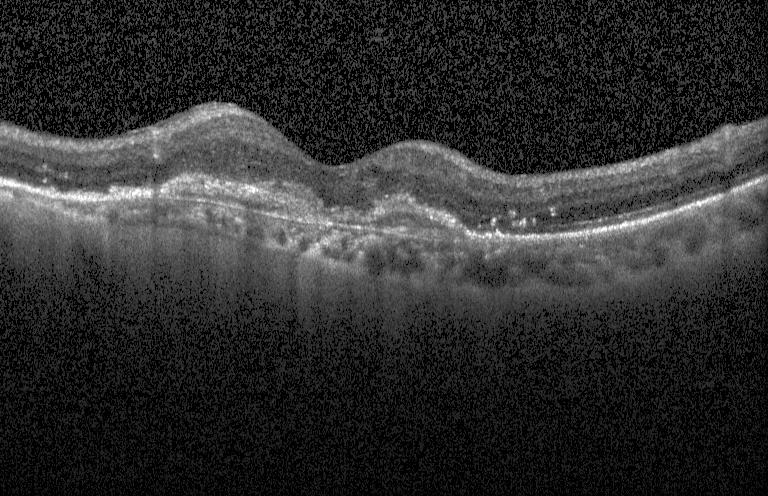 OCT B-scan, SD-OCT
Assessment: CNV.